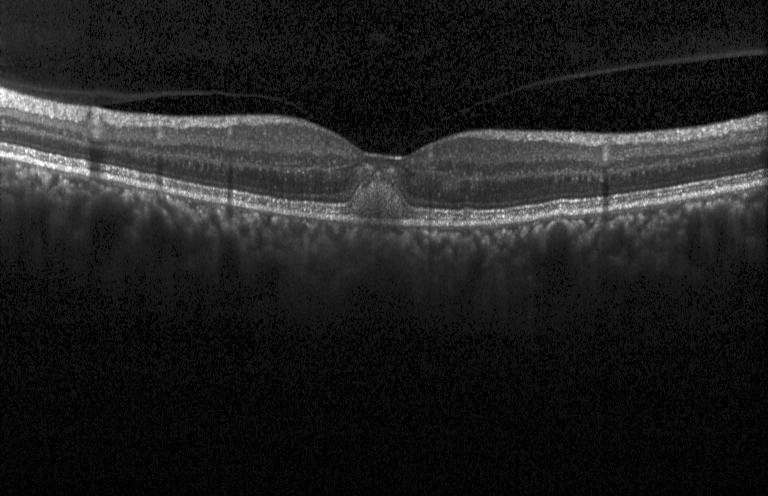

Instrument: Heidelberg Spectralis. Through the macula. Spectral-domain OCT. Optical coherence tomography B-scan.
Macular OCT: choroidal neovascularization (CNV).